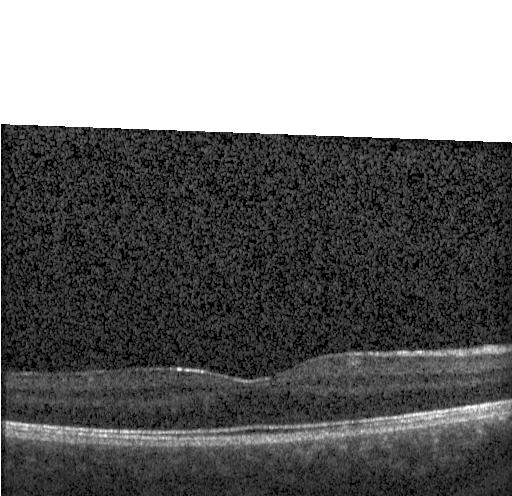 Diagnosis: neither CNV, DME, nor drusen.